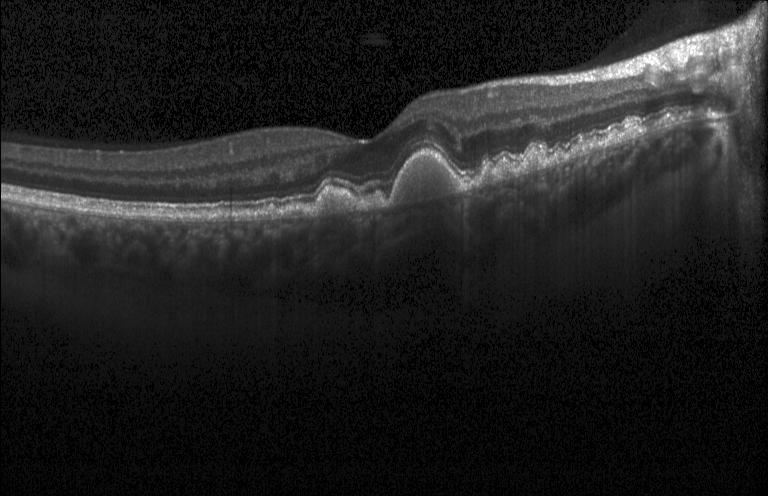
Optical coherence tomography scan
Finding: drusen.